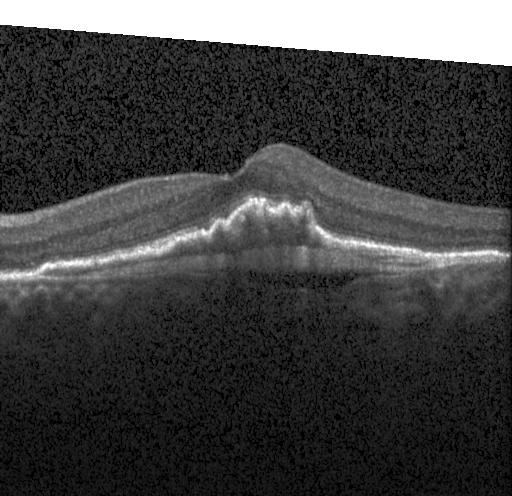
Macular OCT: choroidal neovascularization.